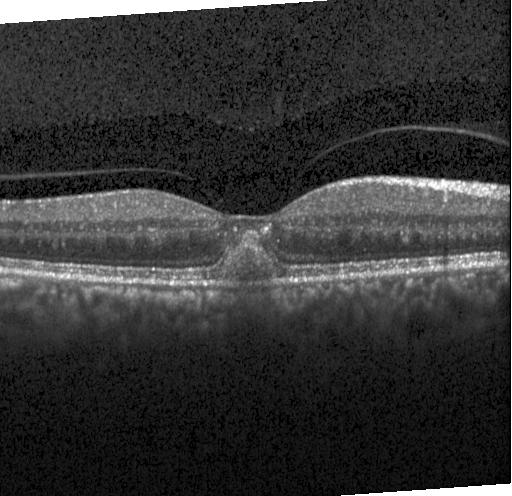

Spectral-domain optical coherence tomography. Fovea-centered. Acquired on a Heidelberg Spectralis. OCT B-scan
Assessment: CNV.